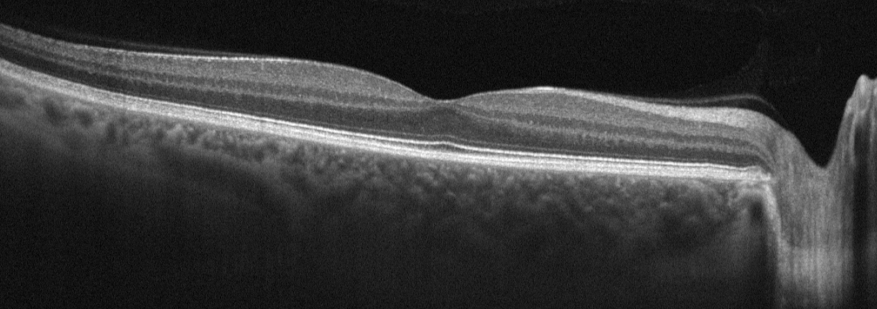 Retinal OCT cross-section — Impression: no evidence of AMD, DME, ERM, RAO, RVO, or VID.